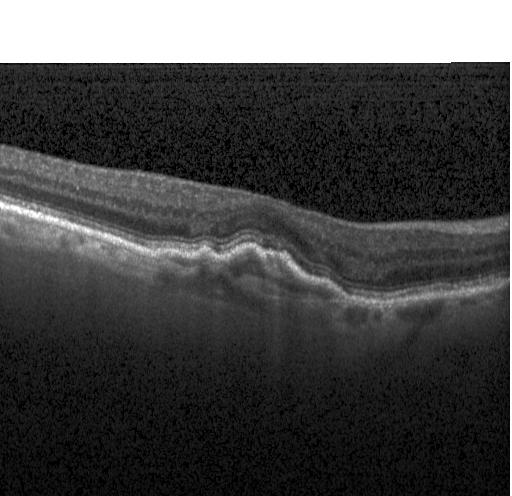
OCT line scan · spectral-domain OCT.
The scan shows a choroidal neovascular membrane.